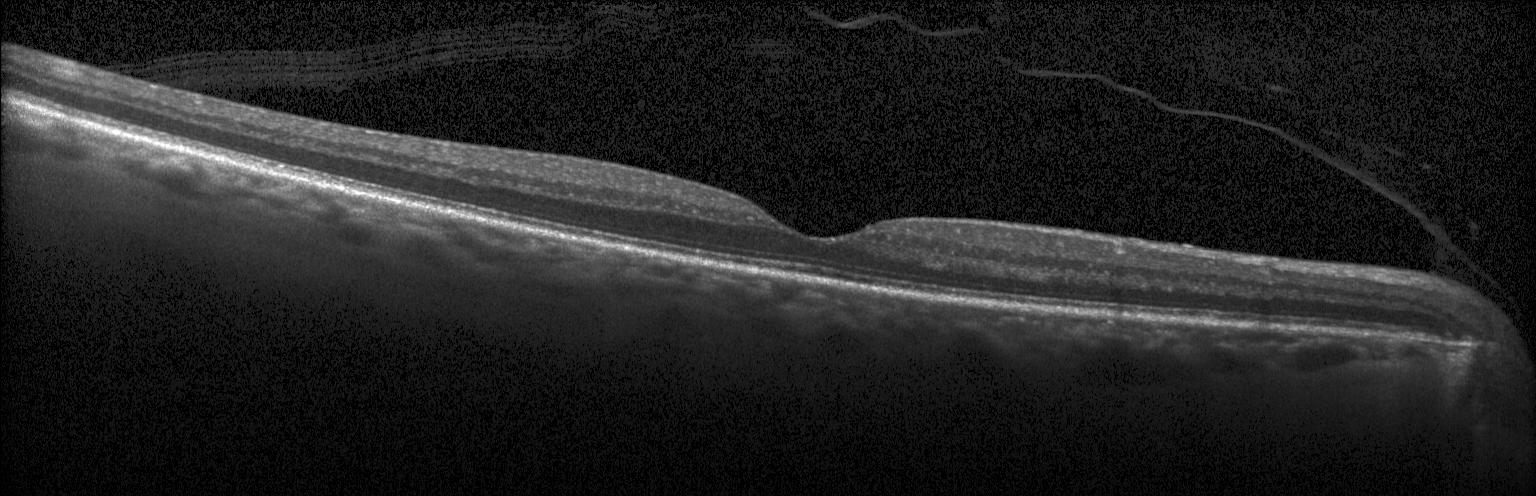

OCT line scan
Assessment: neither choroidal neovascularization, diabetic macular edema, nor drusen.